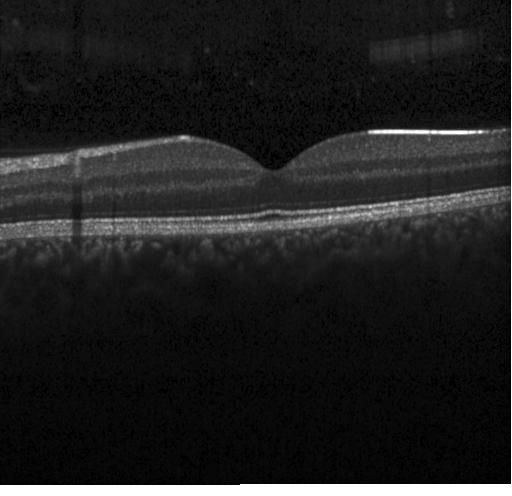

Retinal OCT cross-section
Diagnosis: no evidence of CNV, DME, or drusen.